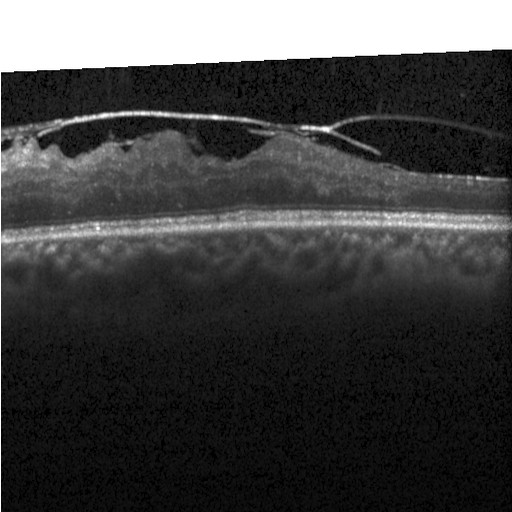
Heidelberg Spectralis. Optical coherence tomography scan
Finding: diabetic macular edema (DME).